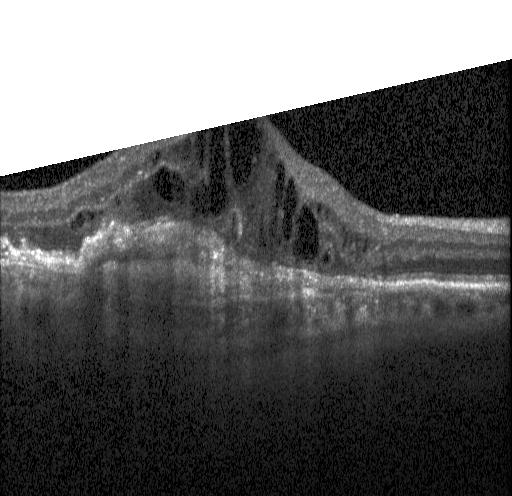

Assessment: choroidal neovascularization.